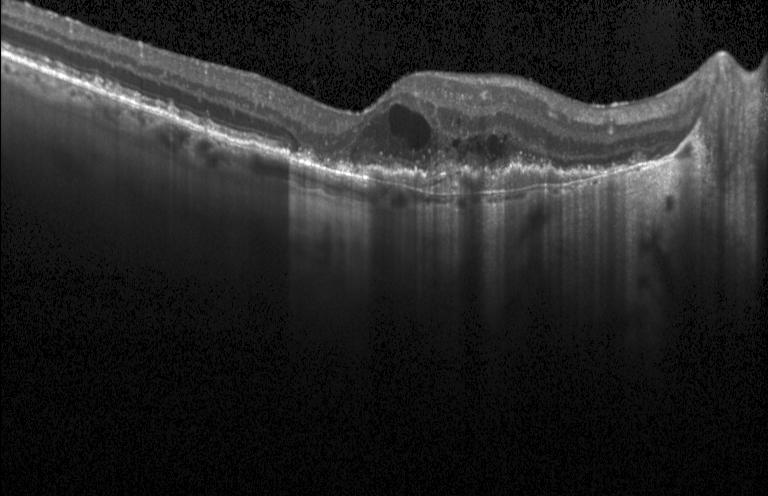
Retinal OCT B-scan; acquired on a Heidelberg Spectralis; horizontal scan through the fovea — Impression: choroidal neovascularization (CNV).